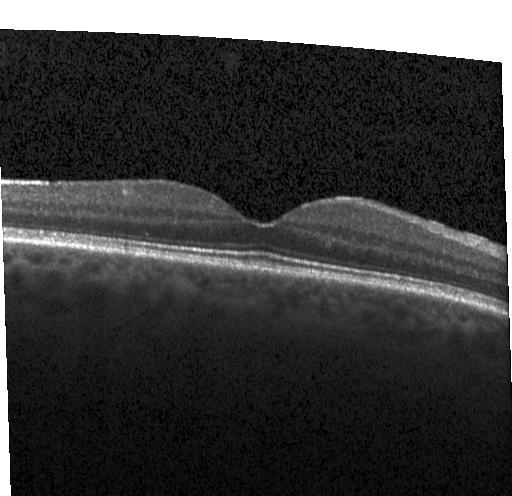
SD-OCT. Macular scan. Optical coherence tomography B-scan. Acquired on a Heidelberg Spectralis.
Dx: no CNV, DME, or drusen.